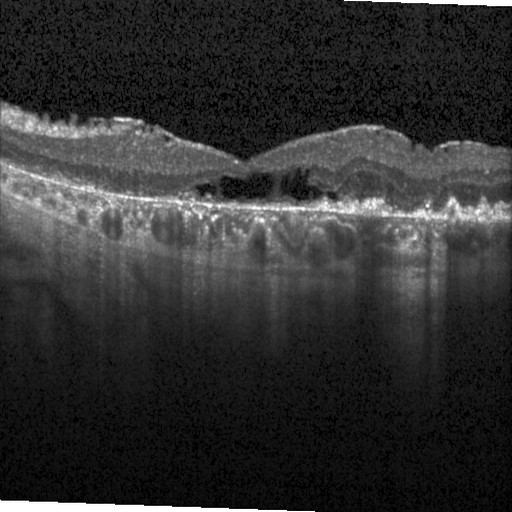 Retinal OCT B-scan, fovea-centered — Diabetic macular edema.